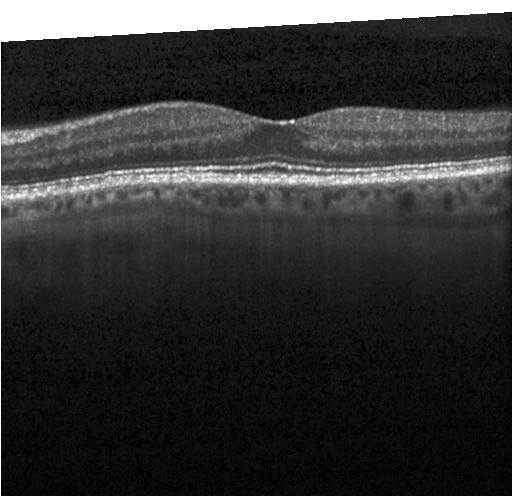
OCT B-scan; Heidelberg Spectralis OCT system; macular scan. Assessment: no CNV, DME, or drusen.